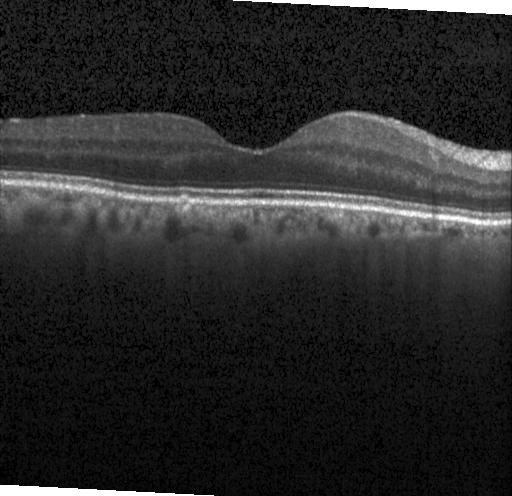

Finding: no CNV, no DME, and no drusen.